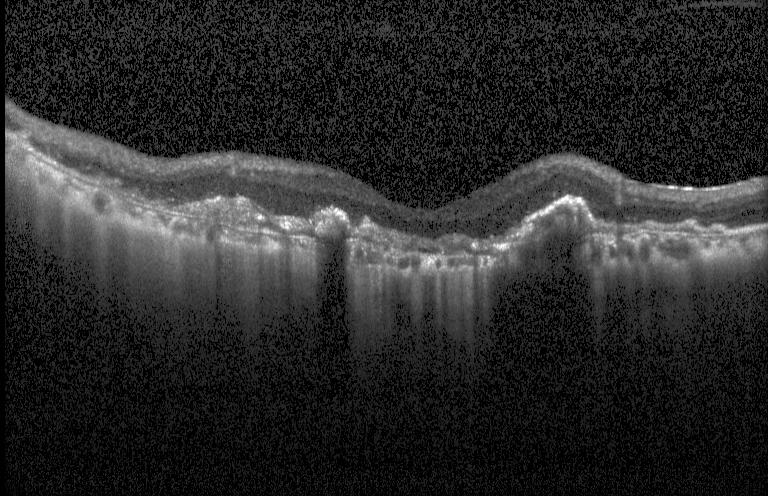
Optical coherence tomography scan; acquired on a Heidelberg Spectralis; spectral-domain optical coherence tomography — Finding: choroidal neovascularization (CNV).